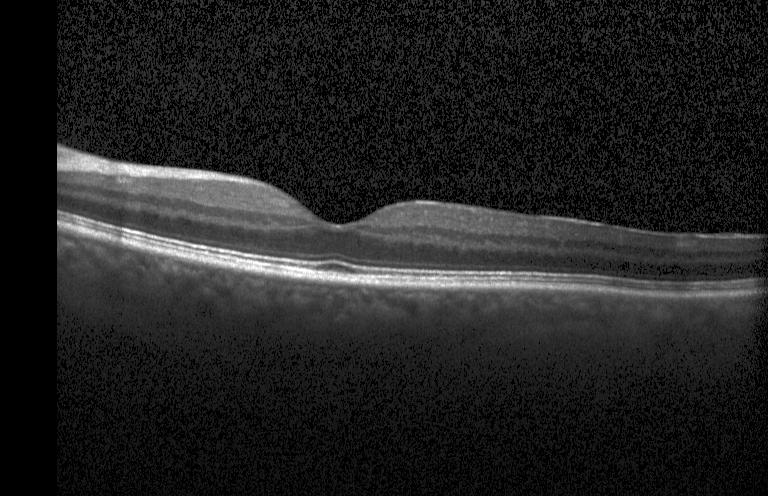
Macular scan · OCT B-scan
Assessment: no evidence of CNV, DME, or drusen.